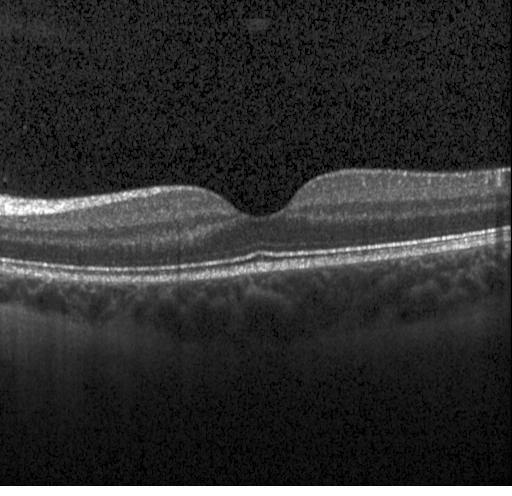 Finding: no CNV, no DME, and no drusen.